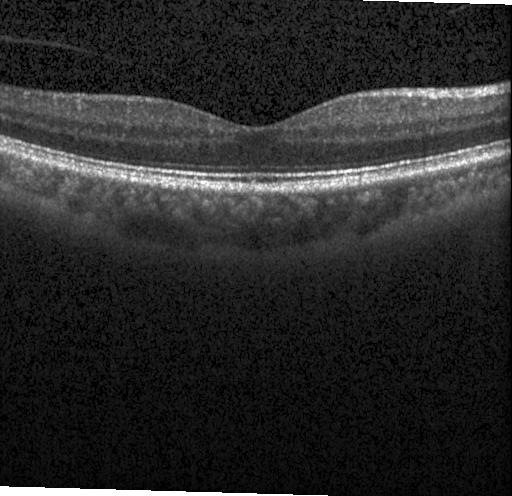 Macular OCT: no evidence of CNV, DME, or drusen.